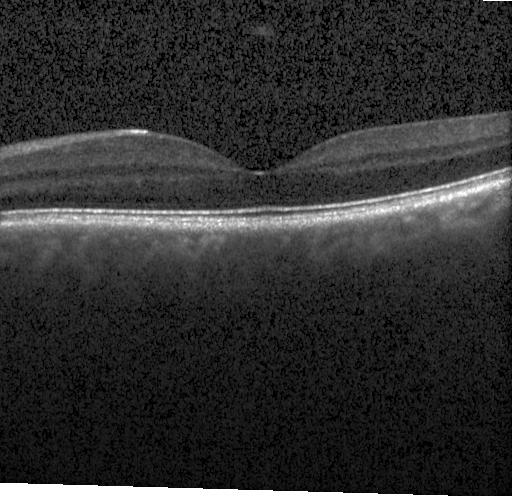

Heidelberg Spectralis · retinal OCT cross-section · SD-OCT.
Impression: no choroidal neovascularization, no diabetic macular edema, and no drusen.